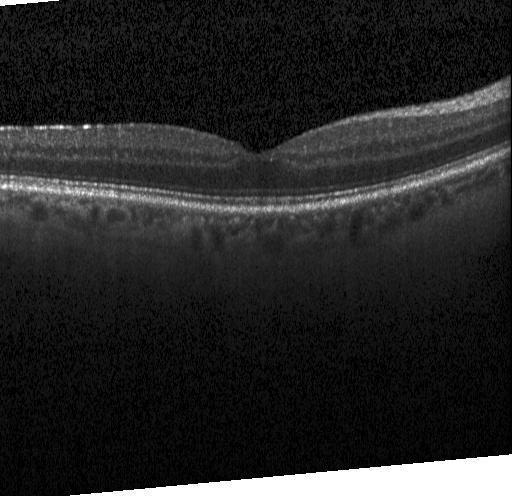

The scan shows no CNV, DME, or drusen.